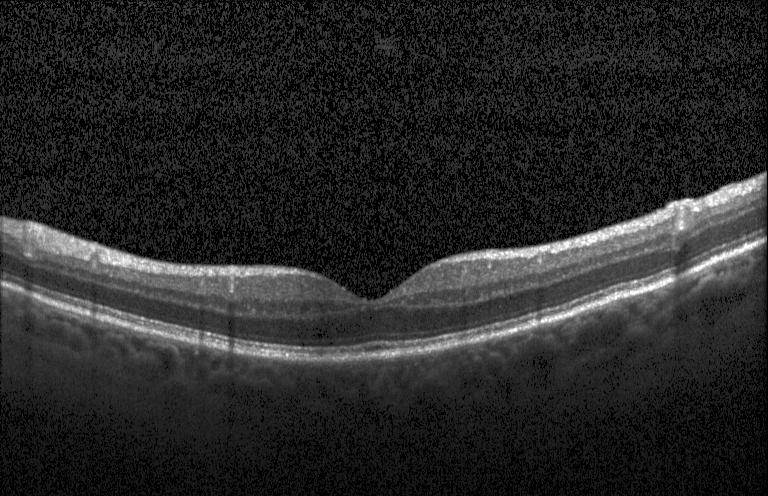
Retinal OCT cross-section showing no evidence of choroidal neovascularization, diabetic macular edema, or drusen.